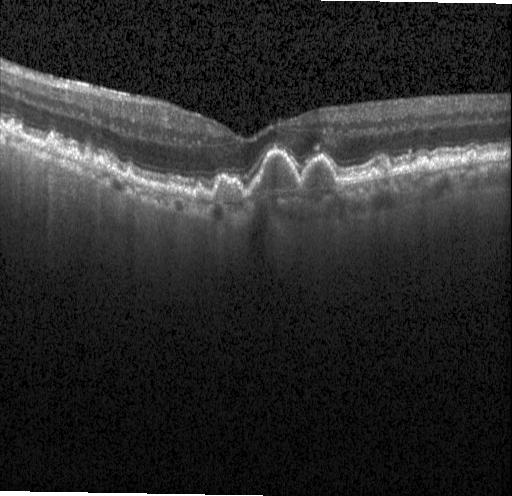 OCT finding: drusen.